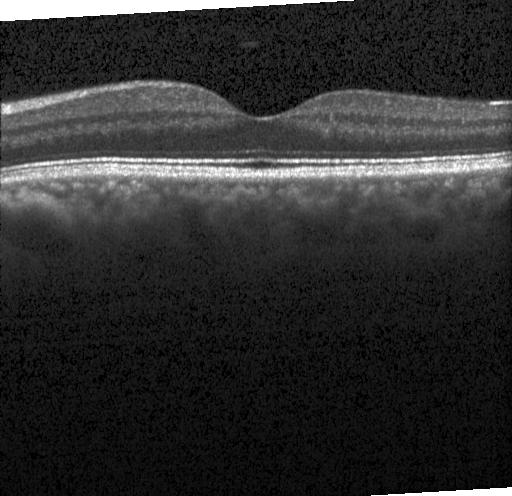 The scan shows neither choroidal neovascularization, diabetic macular edema, nor drusen.